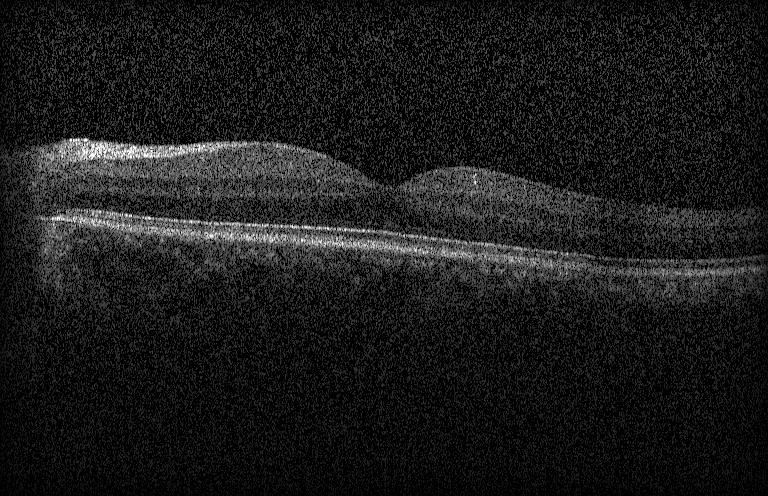 Spectral-domain OCT. Fovea-centered. OCT B-scan. Instrument: Heidelberg Spectralis. Diagnosis: no choroidal neovascularization, diabetic macular edema, or drusen.